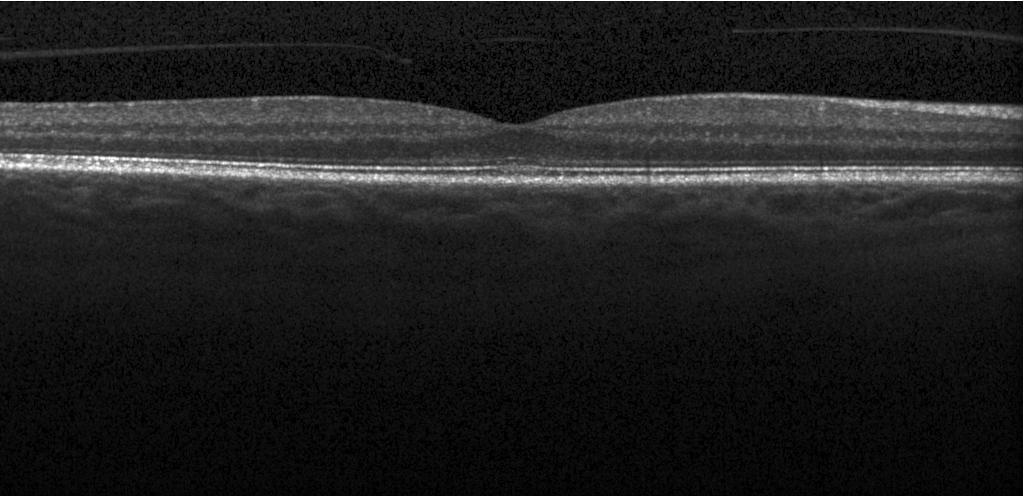

SD-OCT. Acquired on a Heidelberg Spectralis. Fovea-centered. Optical coherence tomography scan.
Finding: no evidence of CNV, DME, or drusen.